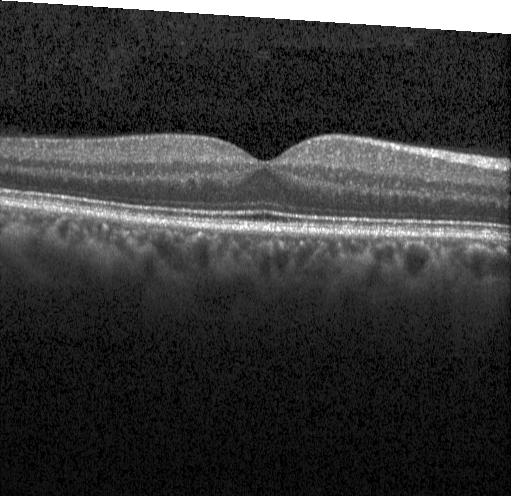

OCT B-scan
Impression: neither choroidal neovascularization, diabetic macular edema, nor drusen.